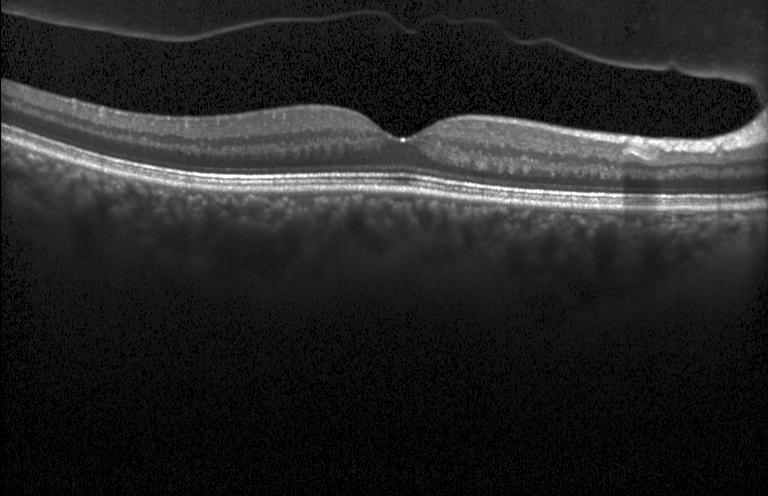

Horizontal scan through the fovea · retinal OCT cross-section · spectral-domain OCT — The scan shows no CNV, no DME, and no drusen.